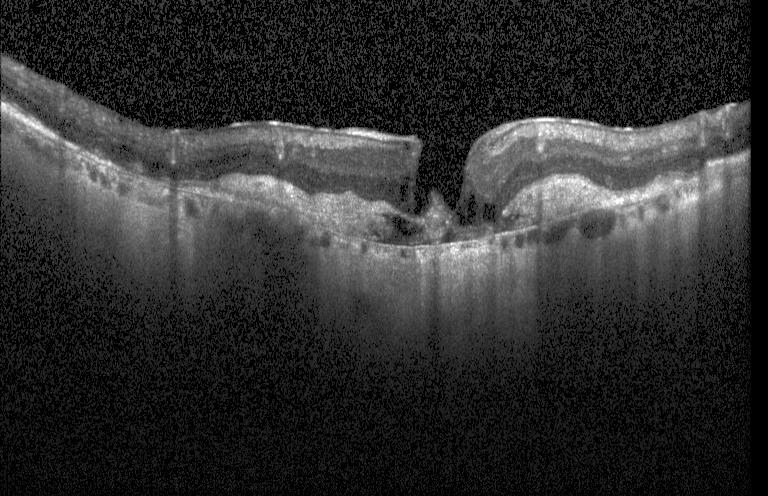

The scan shows a choroidal neovascular membrane.